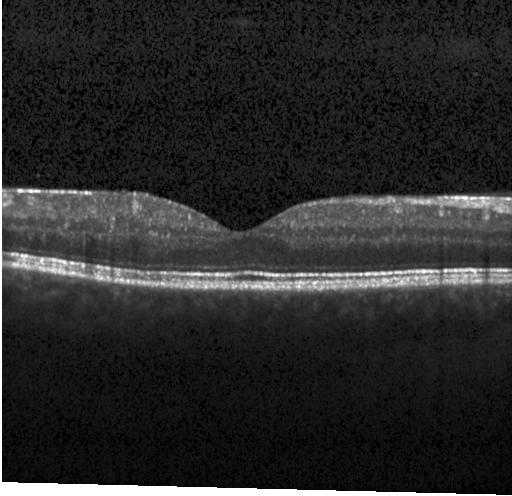

Neither CNV, DME, nor drusen.